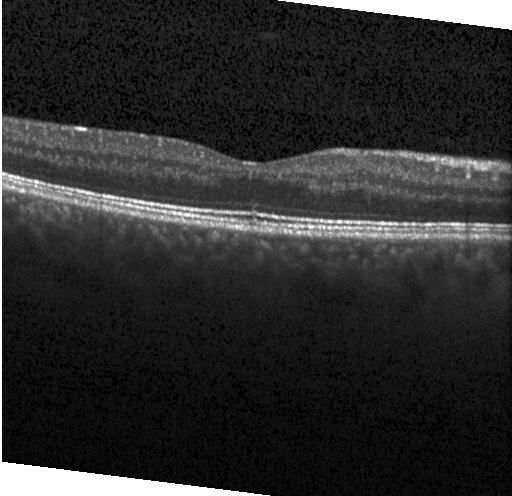 Macular OCT: no evidence of choroidal neovascularization, diabetic macular edema, or drusen.